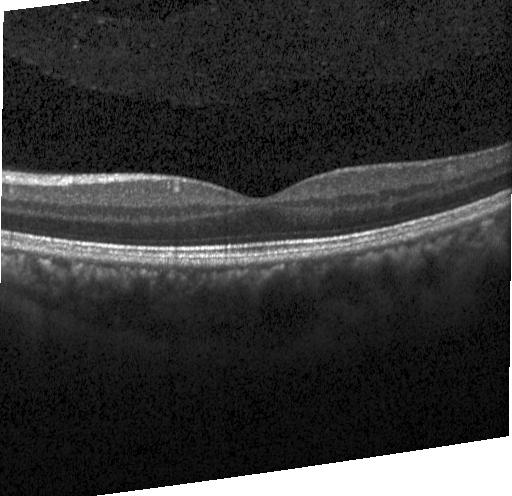
Retinal OCT B-scan — Assessment: neither CNV, DME, nor drusen.